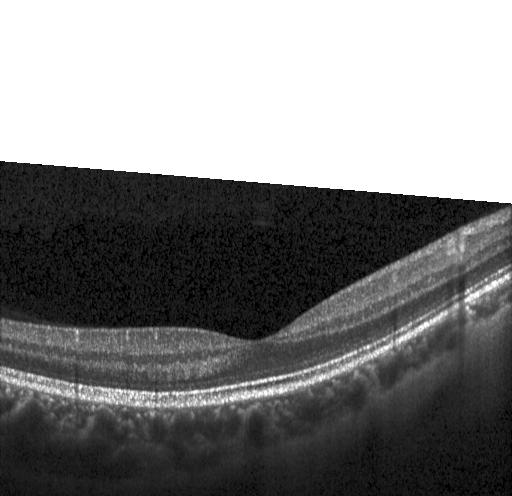 Spectral-domain optical coherence tomography, through the macula, OCT B-scan — OCT finding: no evidence of choroidal neovascularization, diabetic macular edema, or drusen.